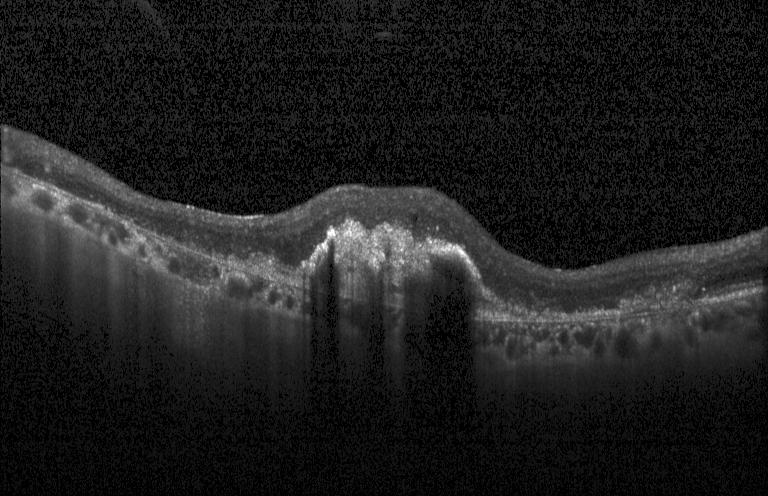

Retinal OCT cross-section. Diagnosis: a choroidal neovascular membrane.